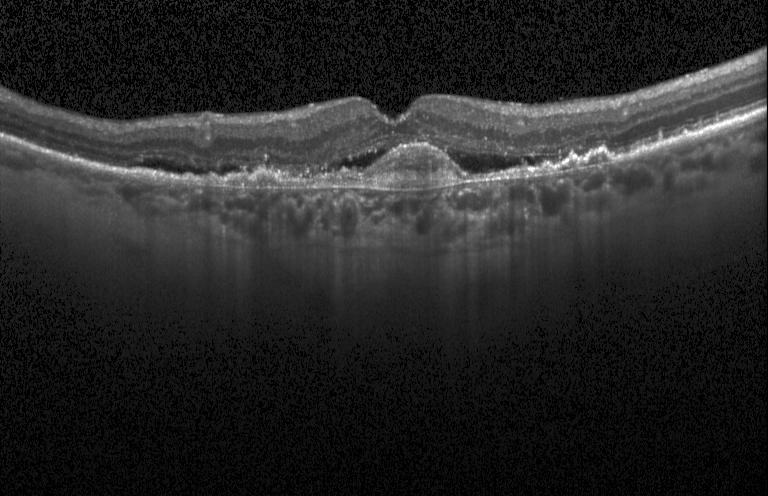
The scan shows choroidal neovascularization (CNV).